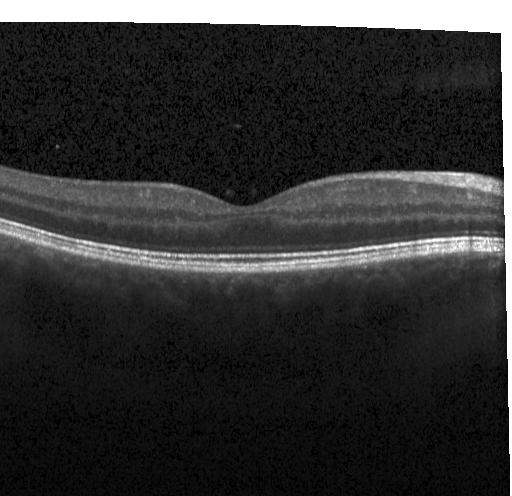
OCT line scan, fovea-centered, acquired on a Heidelberg Spectralis — Finding: neither CNV, DME, nor drusen.